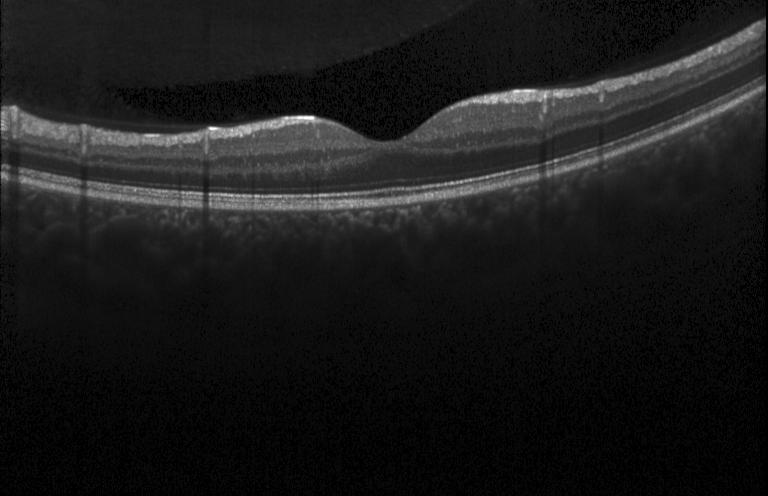
Fovea-centered. Retinal OCT cross-section — The scan shows no evidence of choroidal neovascularization, diabetic macular edema, or drusen.